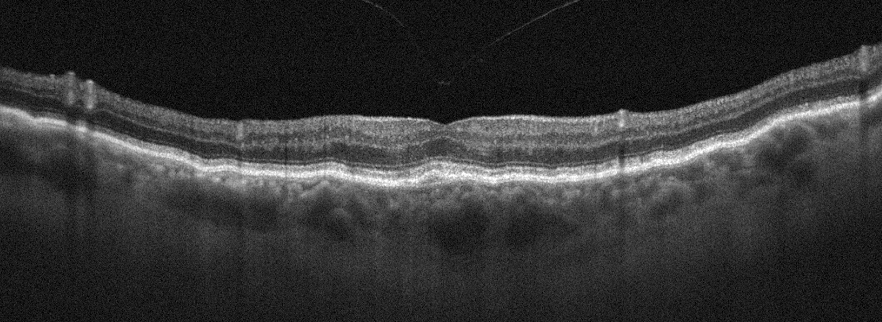
Left eye. Retinal OCT cross-section — Assessment: age-related macular degeneration.